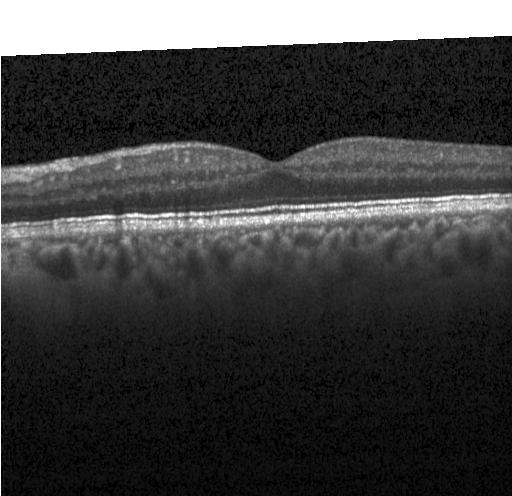 No choroidal neovascularization, no diabetic macular edema, and no drusen.